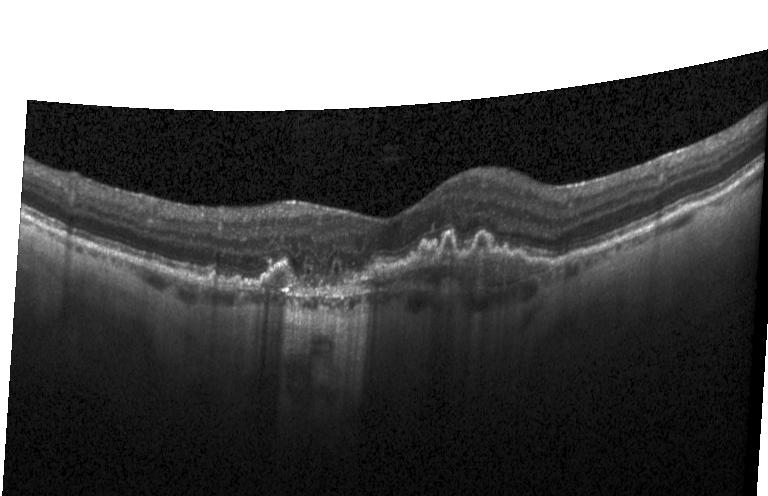

Macular scan. Acquired on a Heidelberg Spectralis. OCT B-scan
Finding: CNV.